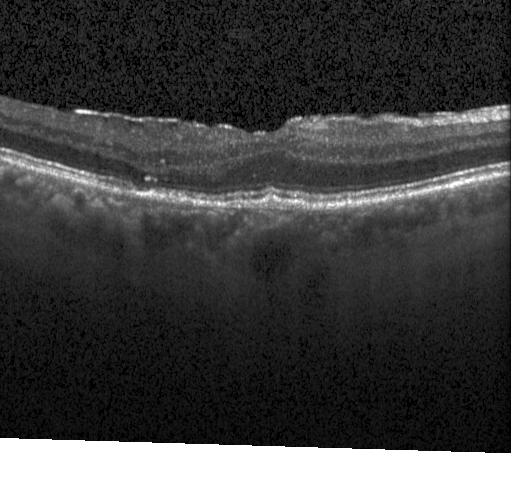
Finding: choroidal neovascularization (CNV).